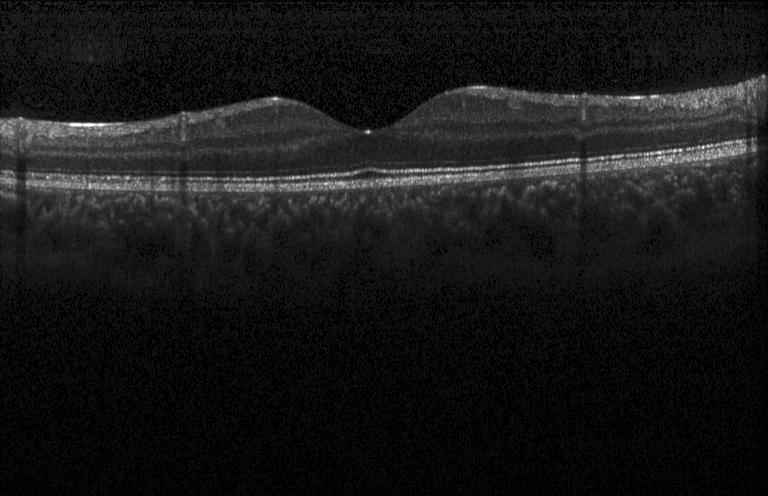
Retinal OCT cross-section — Diagnosis: no evidence of choroidal neovascularization, diabetic macular edema, or drusen.